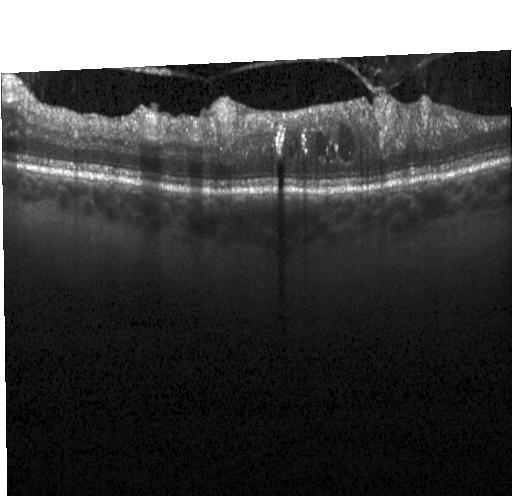 Retinal OCT B-scan · Heidelberg Spectralis · spectral-domain OCT · fovea-centered — Diagnosis: diabetic macular edema (DME).